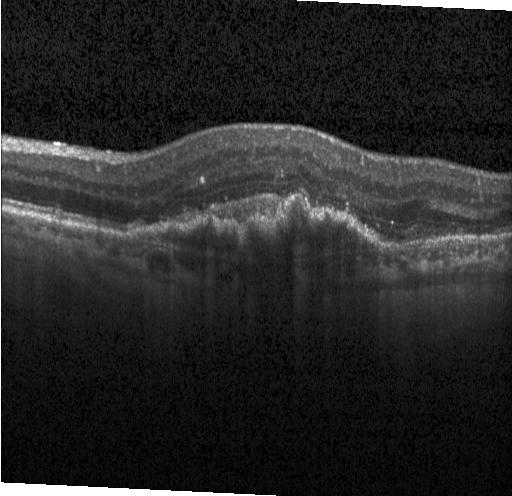
The scan shows CNV.